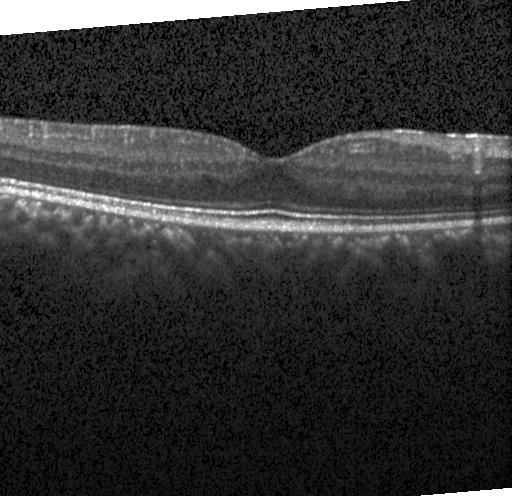 No CNV, DME, or drusen.